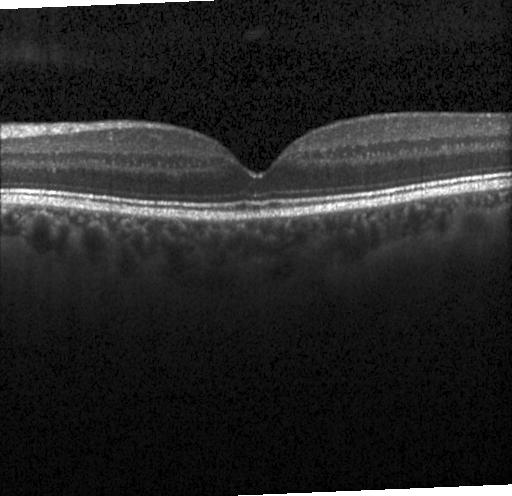

Fovea-centered, retinal OCT B-scan, Heidelberg Spectralis, spectral-domain OCT.
Impression: no CNV, DME, or drusen.